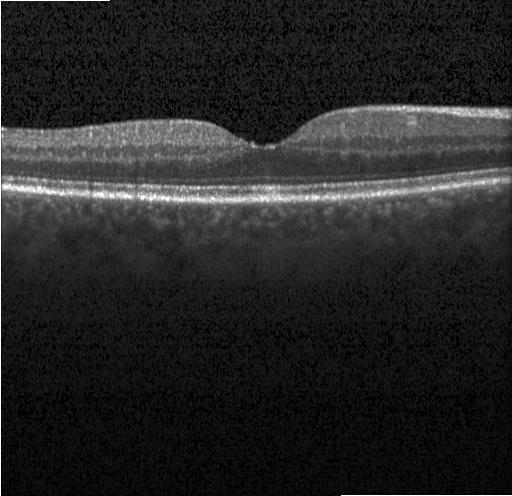
The scan shows no evidence of CNV, DME, or drusen.